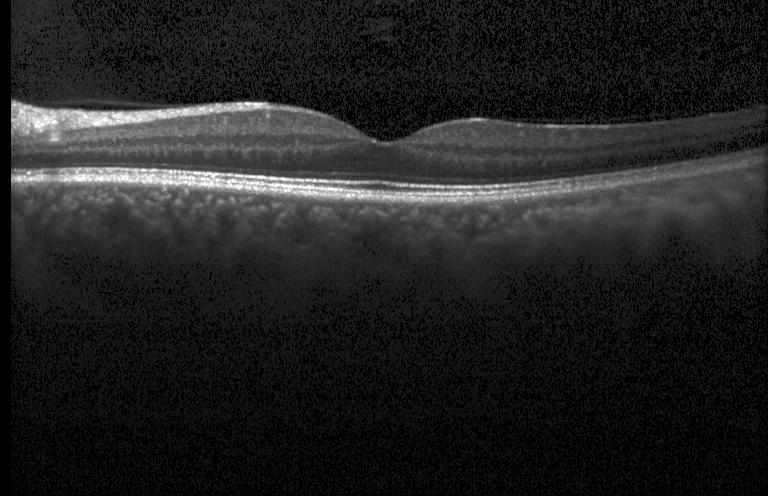 OCT finding: no choroidal neovascularization, no diabetic macular edema, and no drusen.